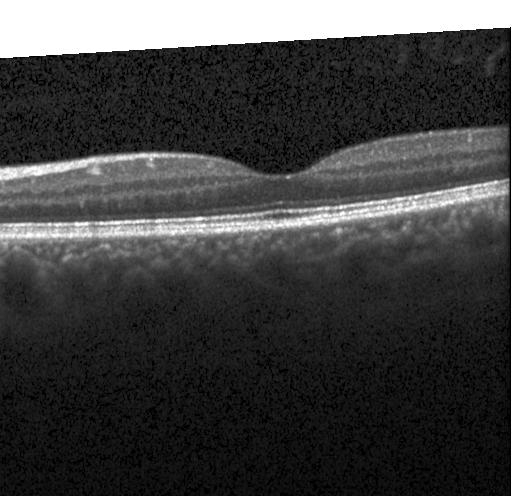 Macular OCT demonstrating no evidence of choroidal neovascularization, diabetic macular edema, or drusen.